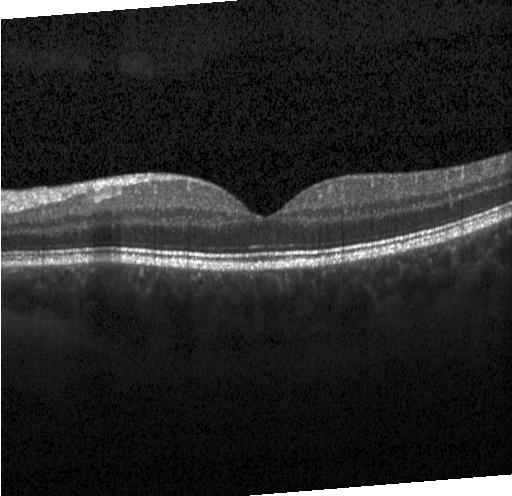
Assessment: no evidence of choroidal neovascularization, diabetic macular edema, or drusen.